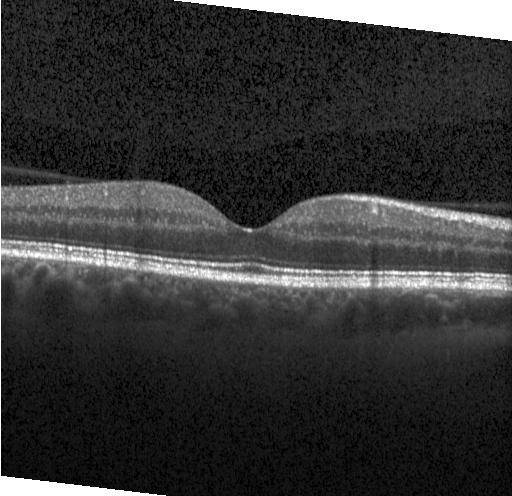

Impression: no choroidal neovascularization, diabetic macular edema, or drusen.